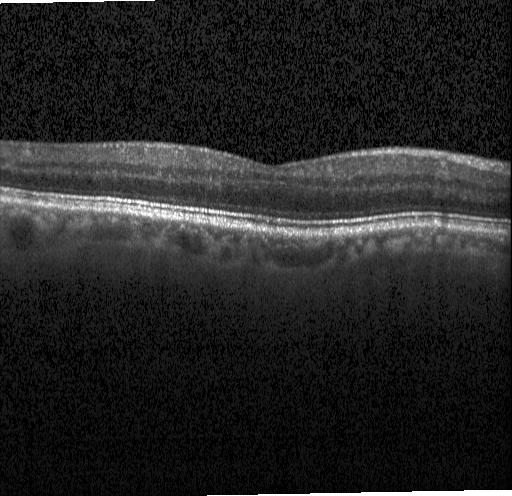
Spectral-domain optical coherence tomography · through the macula · optical coherence tomography scan.
Neither choroidal neovascularization, diabetic macular edema, nor drusen.